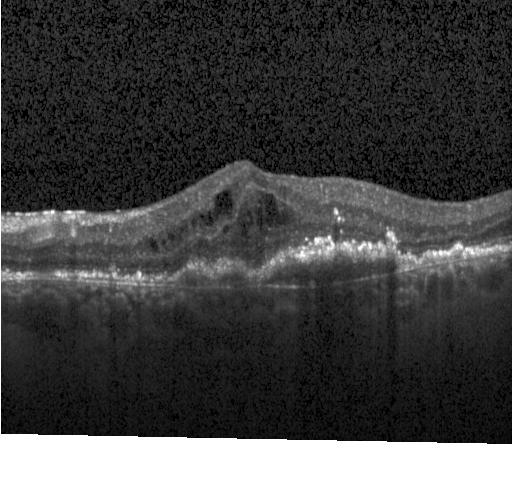
Diagnosis: choroidal neovascularization.